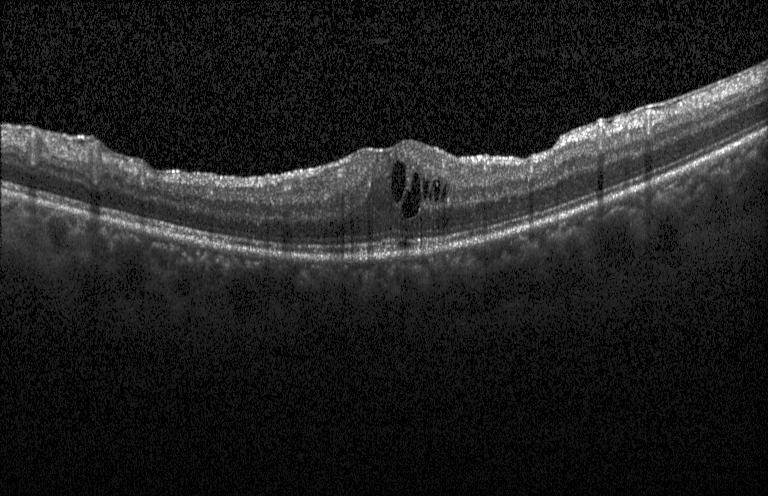
Impression: diabetic macular edema.